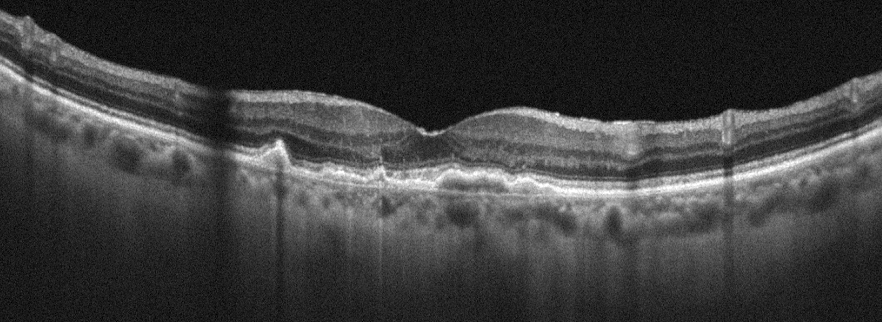

Optical coherence tomography scan · oculus dexter. Age-related macular degeneration (AMD).